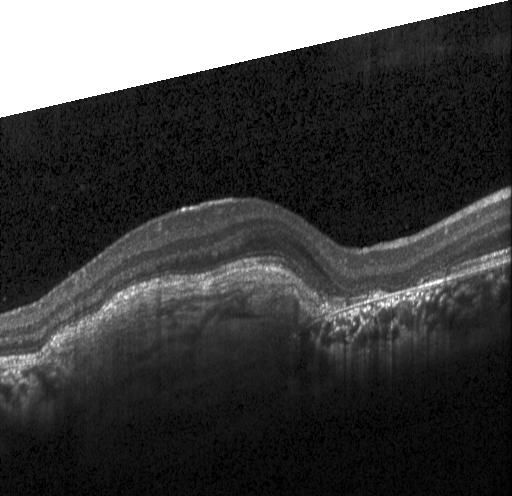
Retinal OCT B-scan · horizontal scan through the fovea.
Macular OCT: a choroidal neovascular membrane.